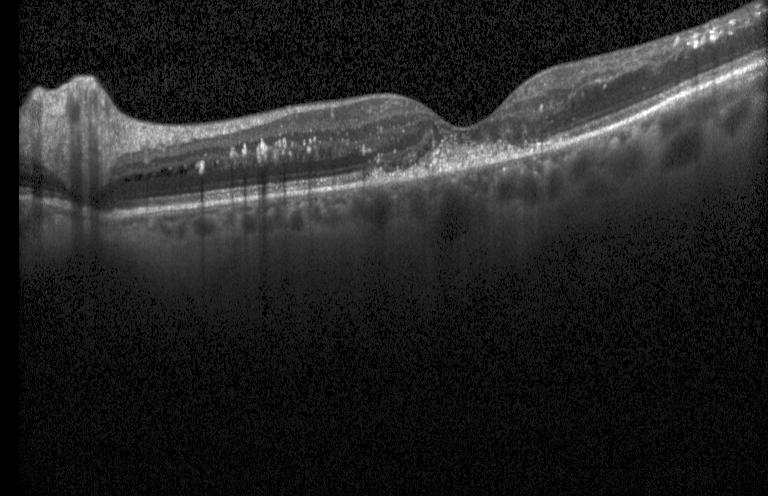 Finding: choroidal neovascularization (CNV).